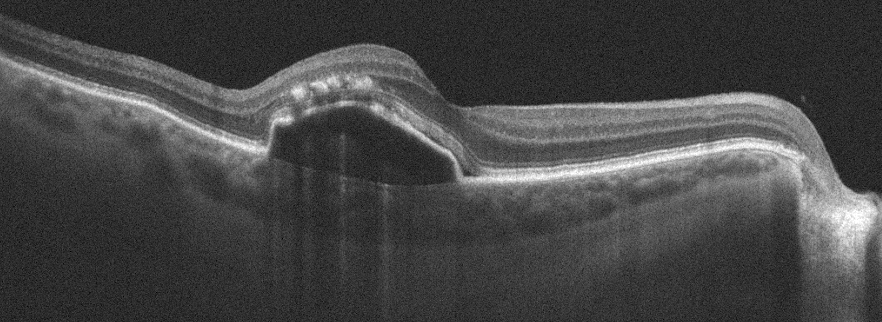
OD · OCT line scan.
Macular OCT: age-related macular degeneration (AMD).